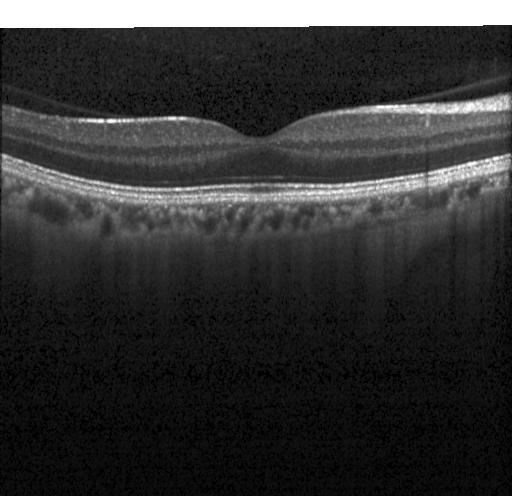

Assessment: no evidence of choroidal neovascularization, diabetic macular edema, or drusen.